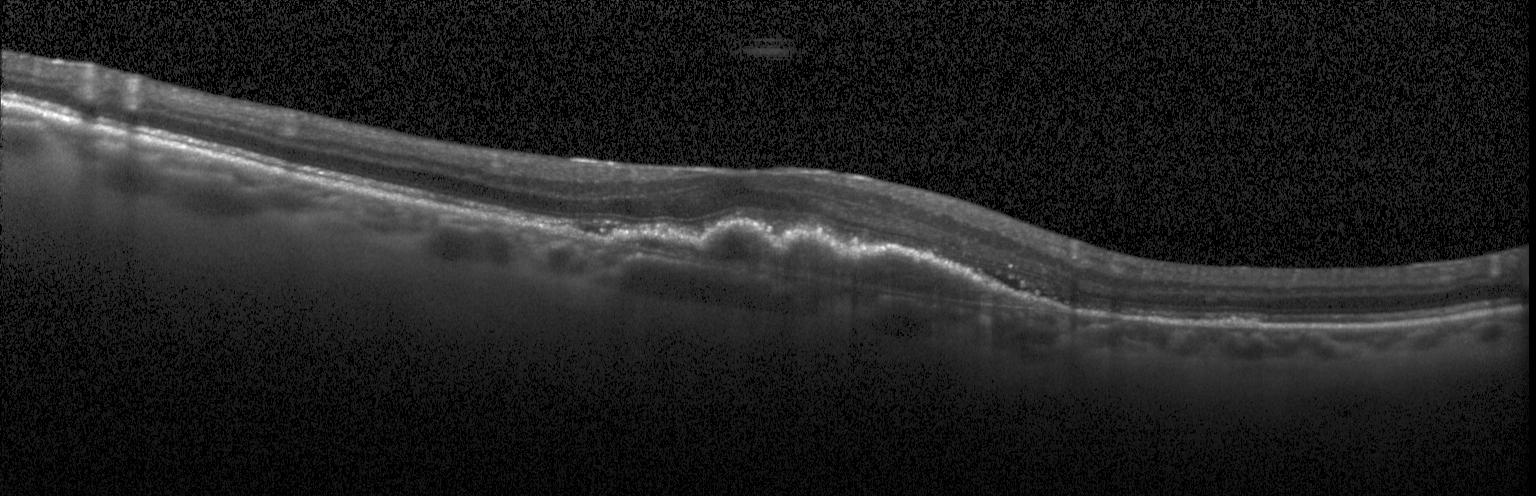
Optical coherence tomography B-scan. Instrument: Heidelberg Spectralis. Spectral-domain OCT.
The scan shows choroidal neovascularization.